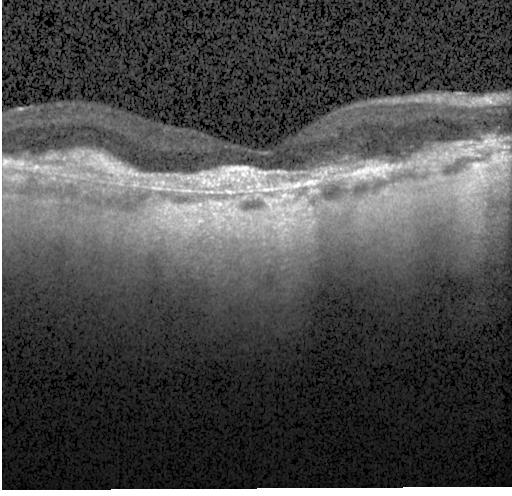 Choroidal neovascularization.